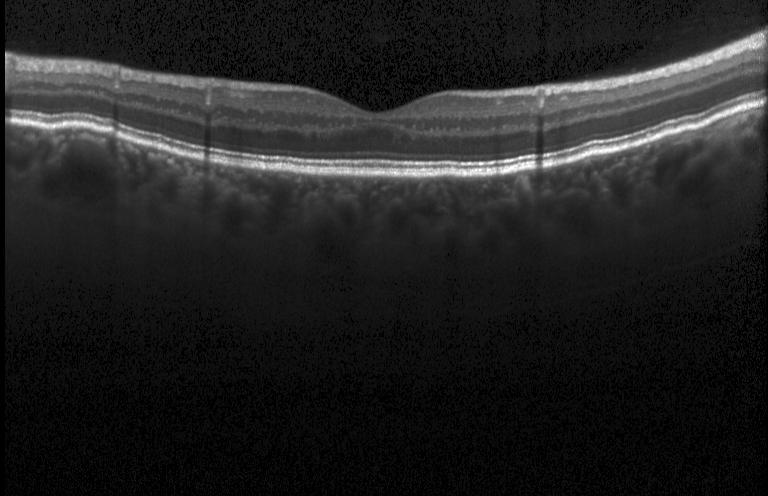
OCT B-scan showing no evidence of CNV, DME, or drusen.